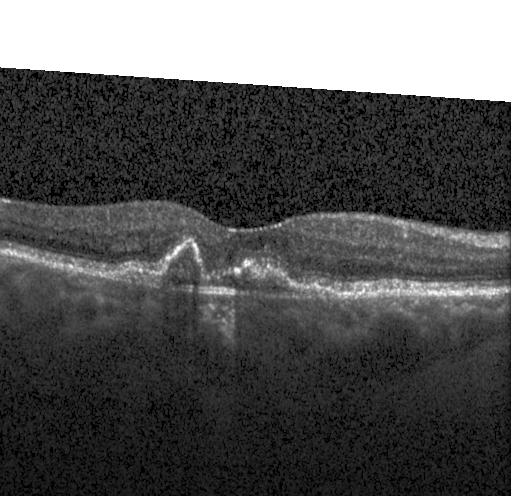
Acquired on a Heidelberg Spectralis; retinal OCT cross-section; spectral-domain OCT; horizontal scan through the fovea
Finding: CNV.